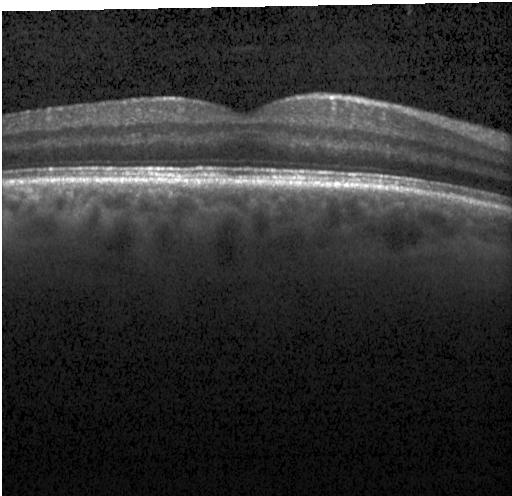

Acquired on a Heidelberg Spectralis · retinal OCT cross-section — Finding: neither choroidal neovascularization, diabetic macular edema, nor drusen.